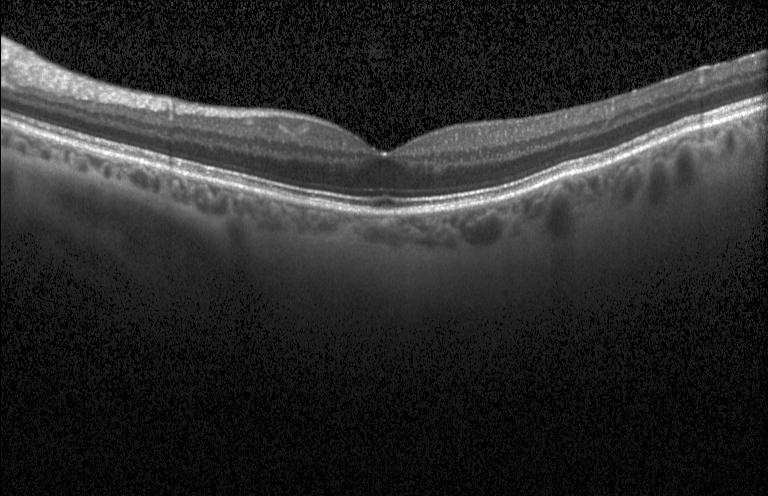 OCT line scan. Horizontal scan through the fovea. Instrument: Heidelberg Spectralis. Assessment: no choroidal neovascularization, no diabetic macular edema, and no drusen.